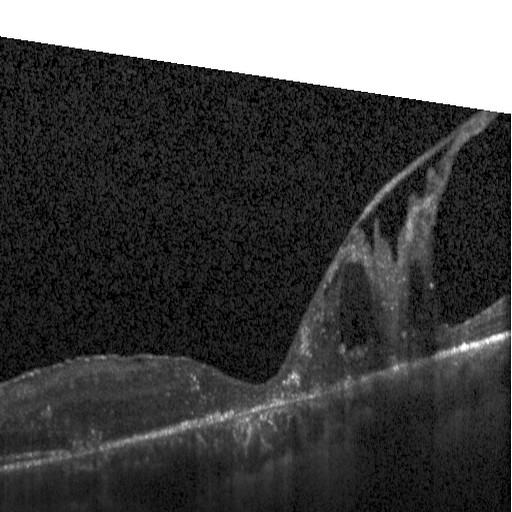
Acquired on a Heidelberg Spectralis; OCT B-scan — This B-scan demonstrates diabetic macular edema.